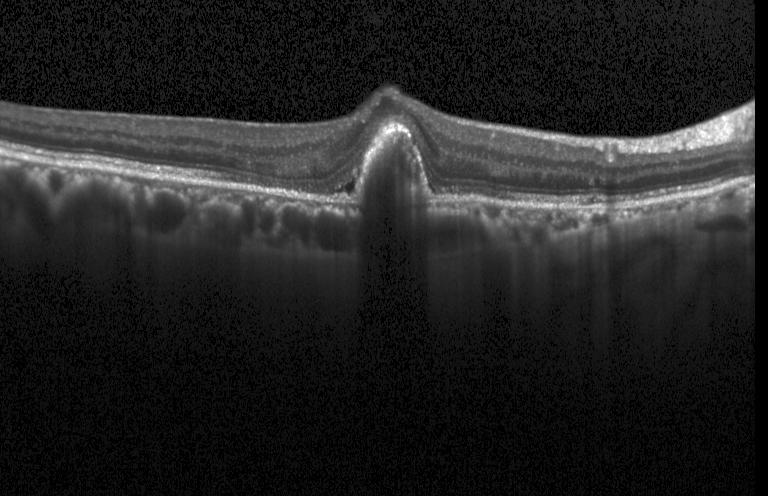
Fovea-centered. Retinal OCT cross-section
Diagnosis: choroidal neovascularization (CNV).